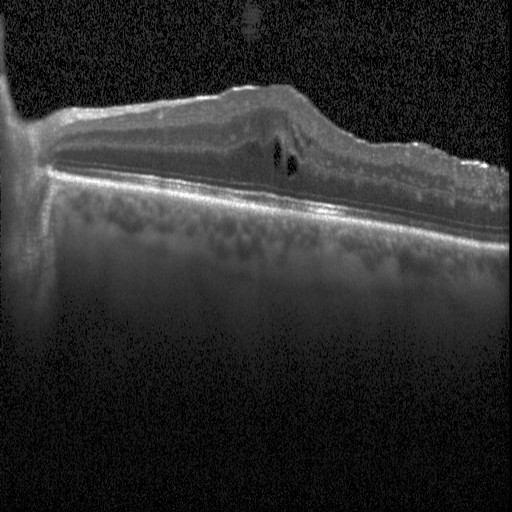 Dx: diabetic macular edema.